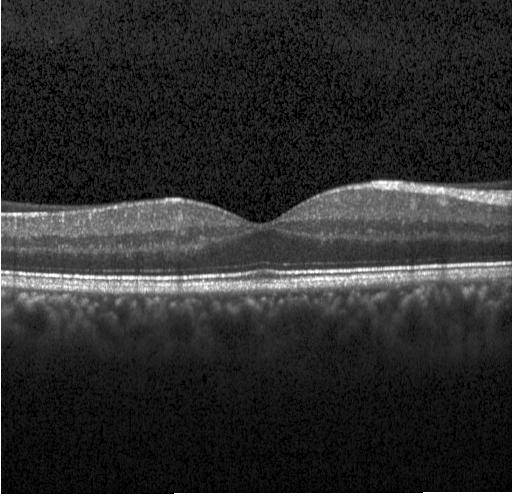
Retinal OCT B-scan
Diagnosis: no choroidal neovascularization, diabetic macular edema, or drusen.